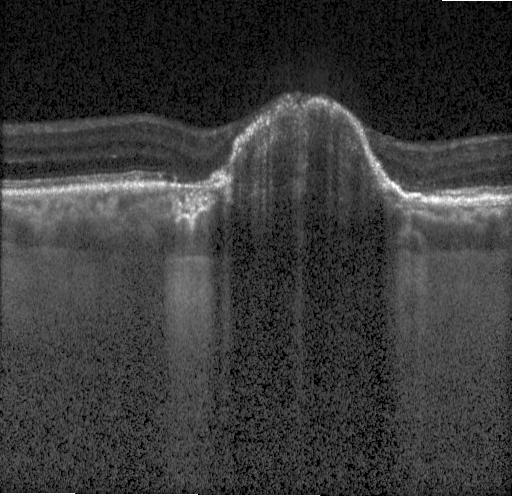 OCT B-scan. A choroidal neovascular membrane.